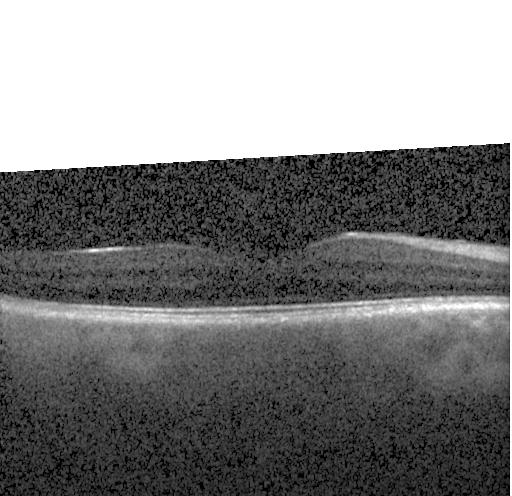
Heidelberg Spectralis OCT system · retinal OCT cross-section · SD-OCT — Finding: no choroidal neovascularization, diabetic macular edema, or drusen.